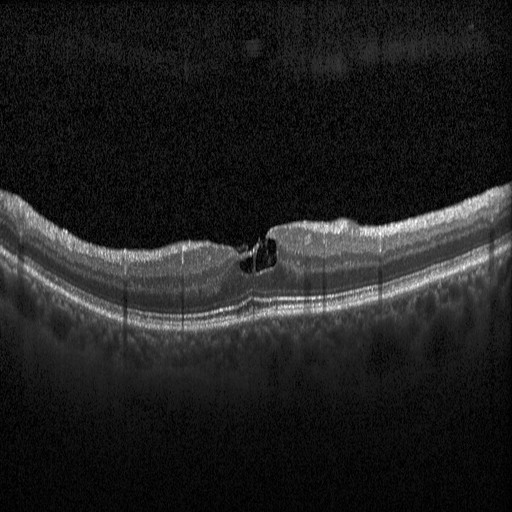

SD-OCT · retinal OCT cross-section — Macular OCT: DME.